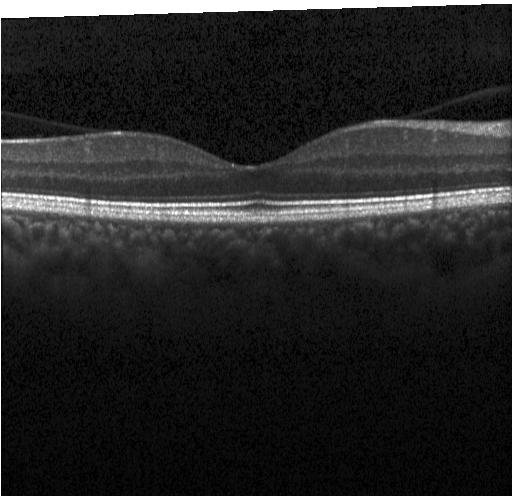

Diagnosis: no evidence of choroidal neovascularization, diabetic macular edema, or drusen.